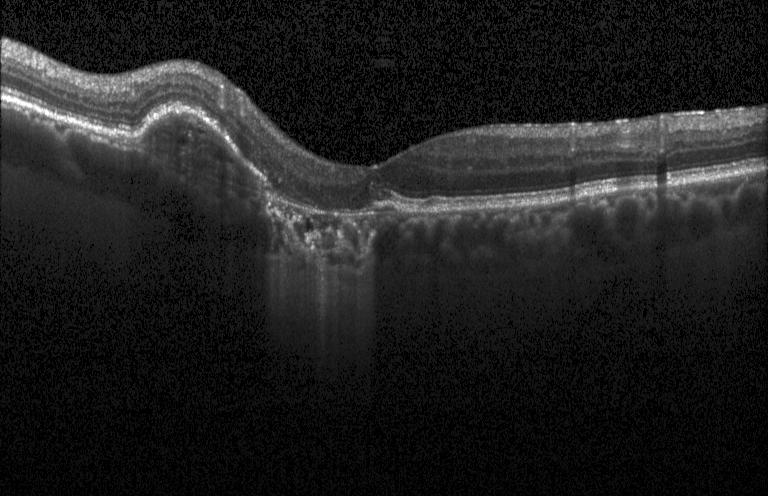 Retinal OCT B-scan — Impression: choroidal neovascularization (CNV).